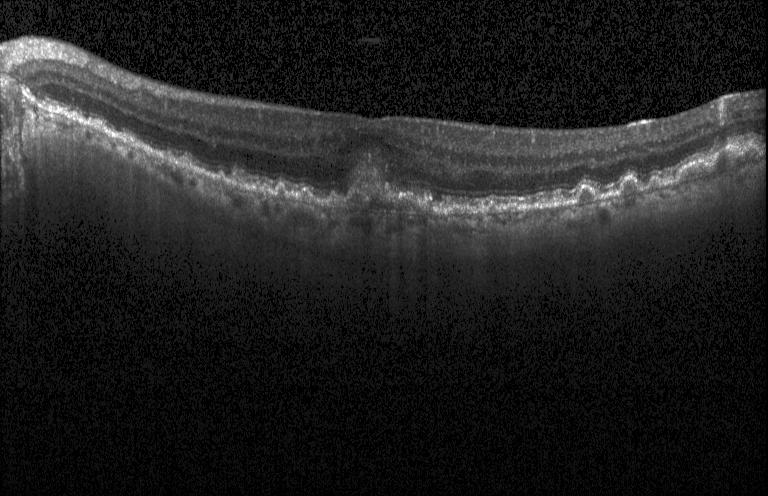 Spectral-domain optical coherence tomography · retinal OCT B-scan · acquired on a Heidelberg Spectralis · fovea-centered
Assessment: CNV.